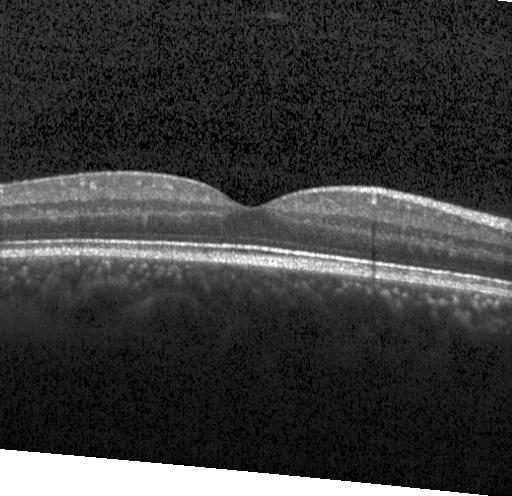
Retinal OCT cross-section; horizontal scan through the fovea. OCT finding: no choroidal neovascularization, no diabetic macular edema, and no drusen.